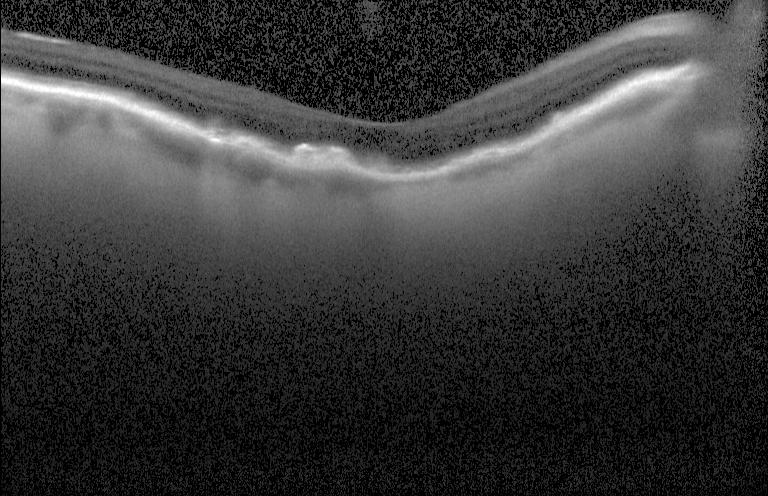

Macular OCT demonstrating choroidal neovascularization (CNV).